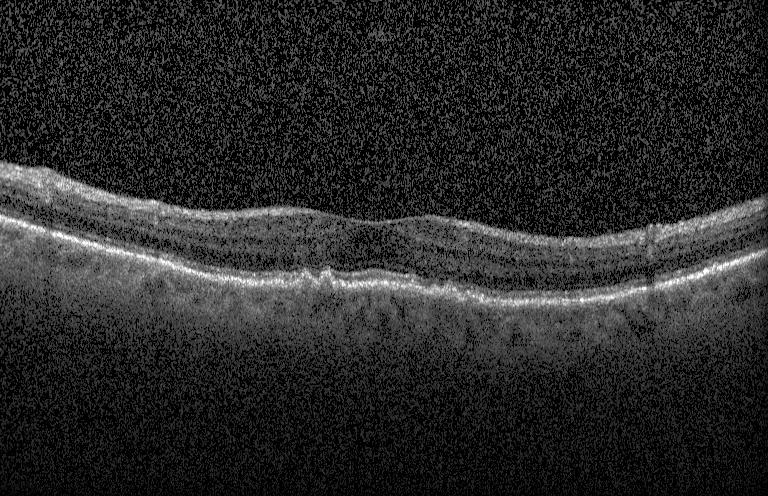
Heidelberg Spectralis; spectral-domain optical coherence tomography; optical coherence tomography B-scan; centered on the fovea.
Finding: sub-RPE drusenoid deposits.